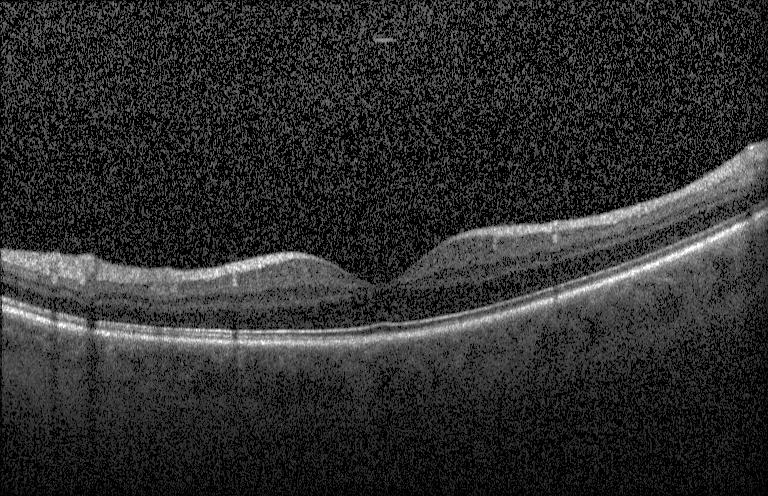 SD-OCT, Heidelberg Spectralis OCT system, retinal OCT B-scan. Finding: neither choroidal neovascularization, diabetic macular edema, nor drusen.